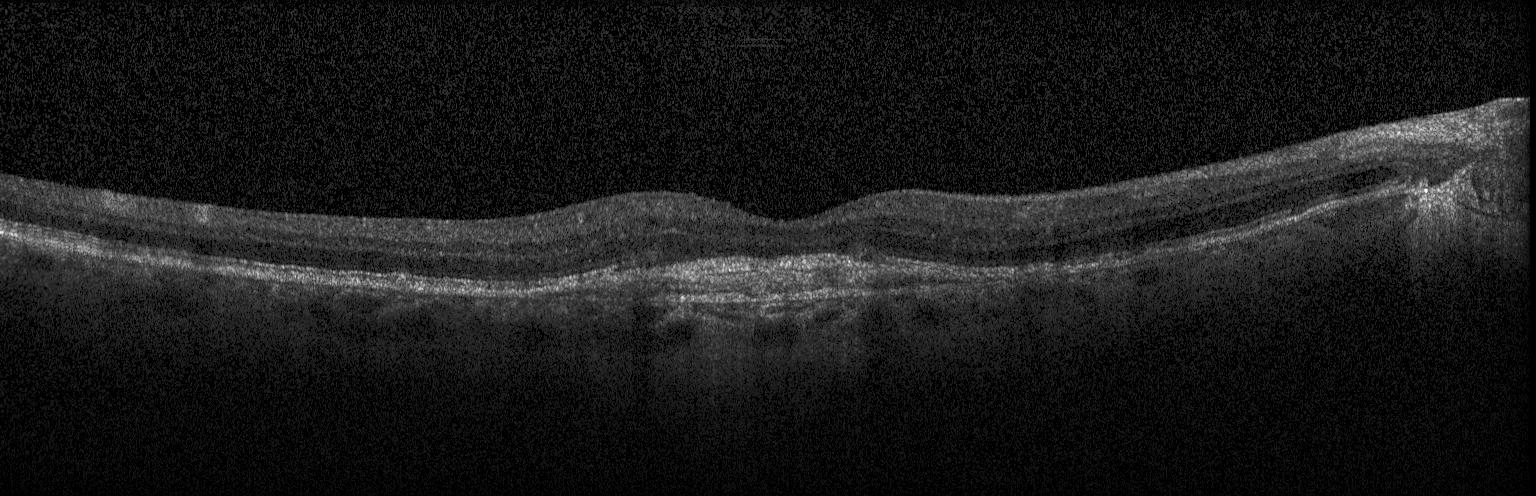

Finding: choroidal neovascularization.